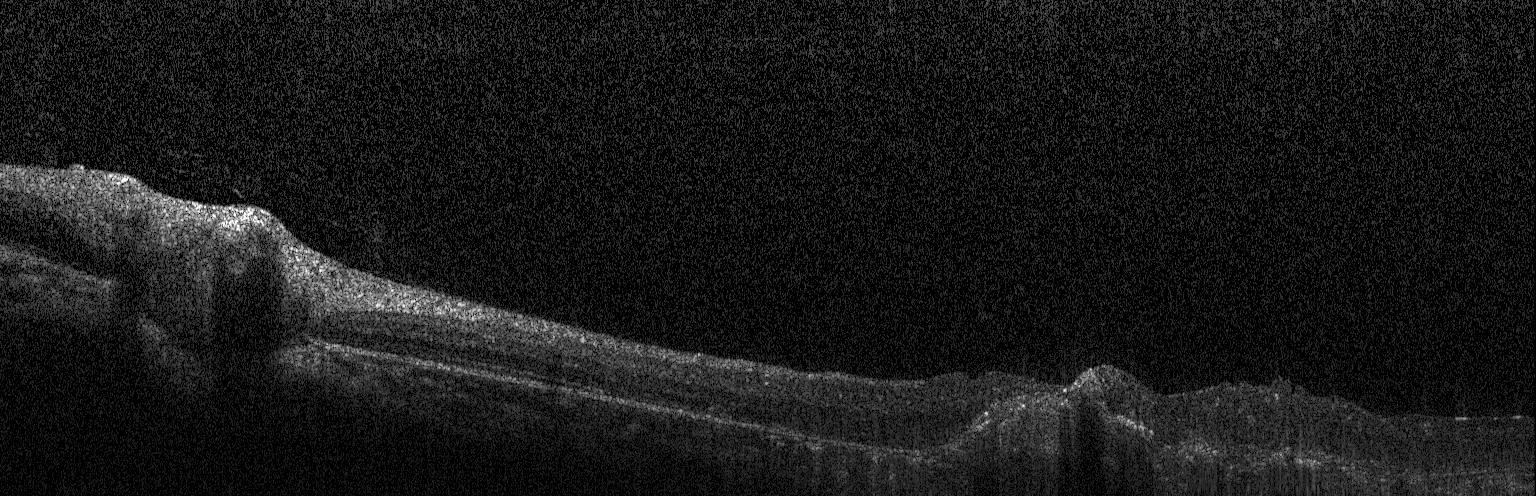
Retinal OCT cross-section showing a choroidal neovascular membrane.